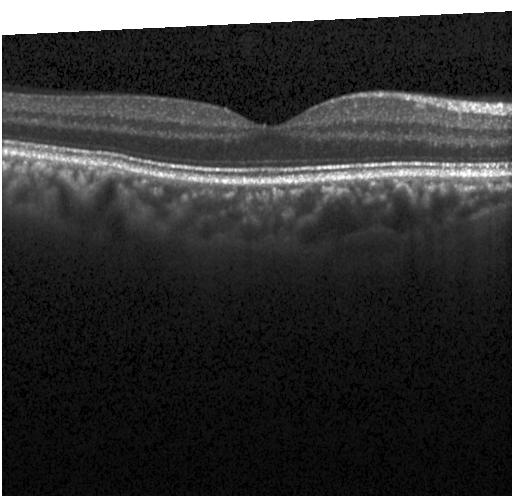

Finding: no choroidal neovascularization, no diabetic macular edema, and no drusen.